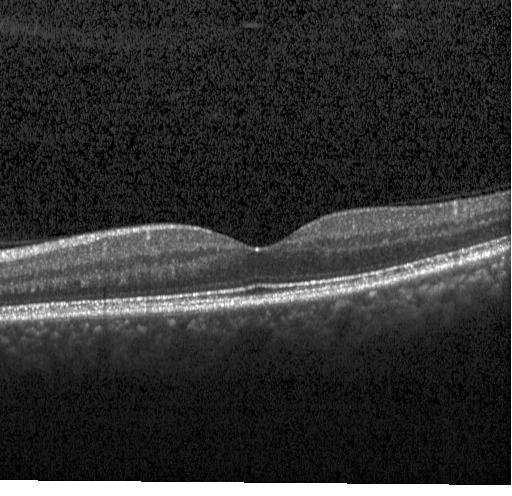
OCT line scan; spectral-domain optical coherence tomography; Heidelberg Spectralis.
Macular OCT: no CNV, no DME, and no drusen.